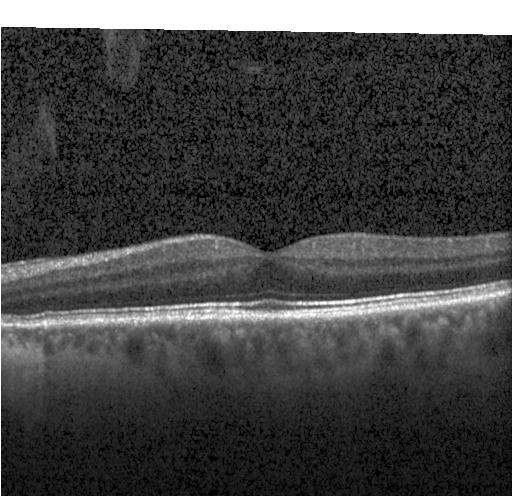

Acquired on a Heidelberg Spectralis. Retinal OCT B-scan. The scan shows neither choroidal neovascularization, diabetic macular edema, nor drusen.